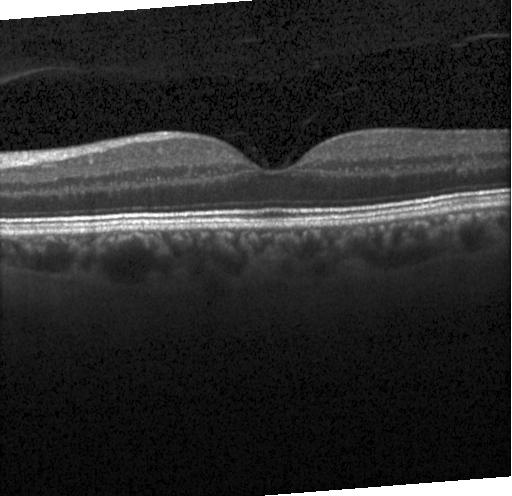

Spectral-domain OCT. OCT line scan. Heidelberg Spectralis. Through the macula.
This B-scan demonstrates no evidence of choroidal neovascularization, diabetic macular edema, or drusen.